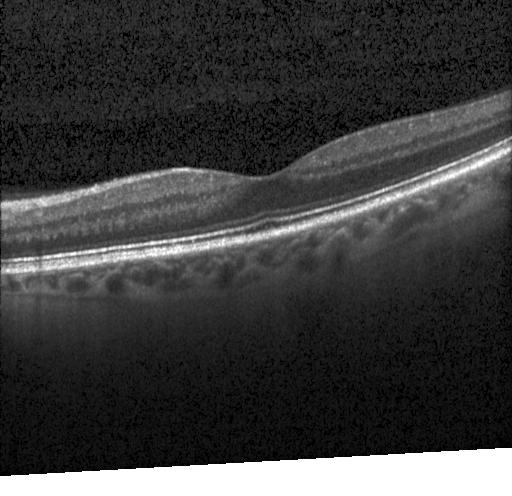

Optical coherence tomography B-scan. Centered on the fovea. Impression: no choroidal neovascularization, diabetic macular edema, or drusen.